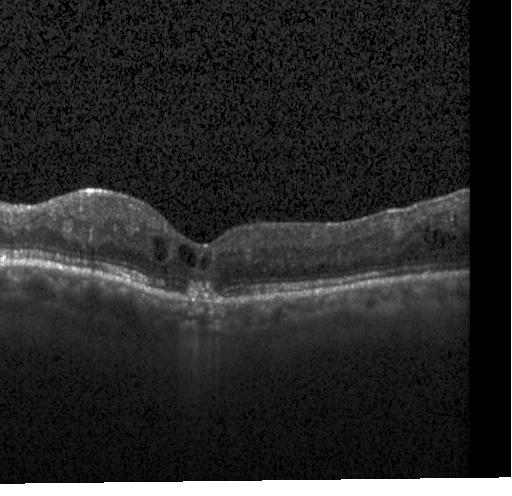
Finding: CNV.